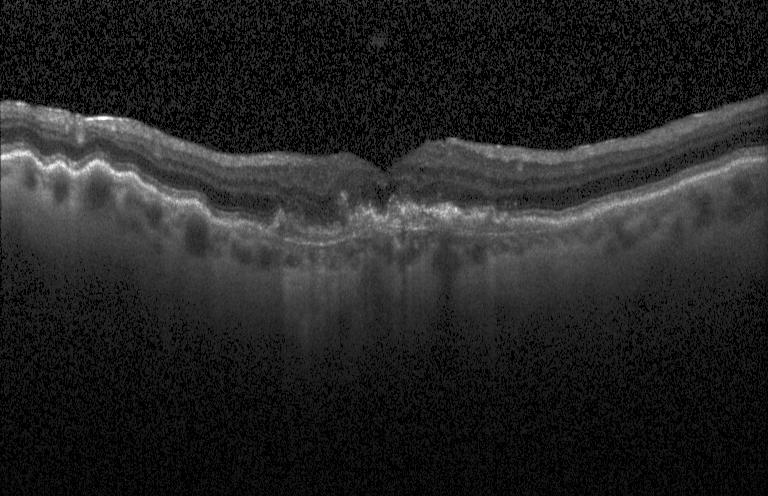 OCT B-scan · acquired on a Heidelberg Spectralis.
Finding: choroidal neovascularization.